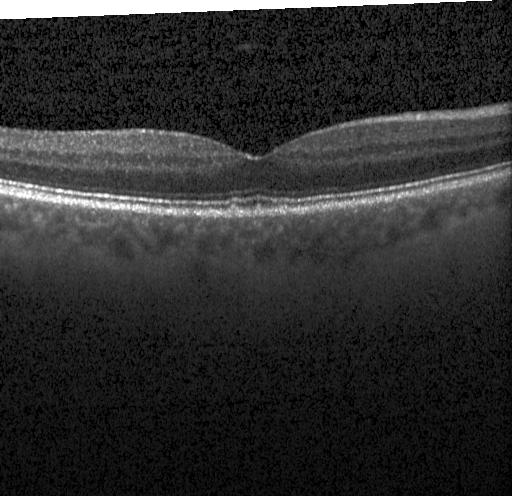

Horizontal scan through the fovea. OCT line scan. SD-OCT
Macular OCT: drusen.